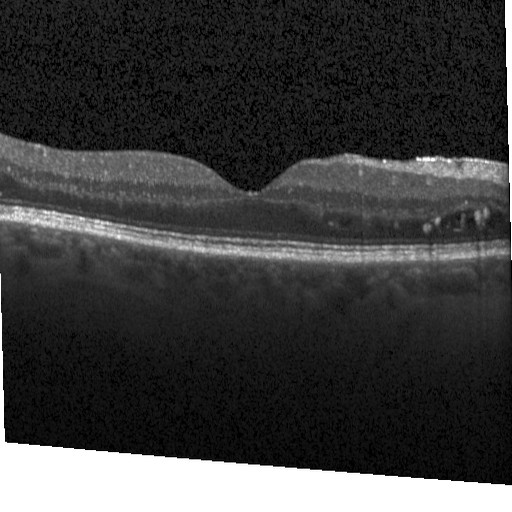

Retinal OCT B-scan; Heidelberg Spectralis OCT system; spectral-domain OCT
Macular OCT: diabetic macular edema.